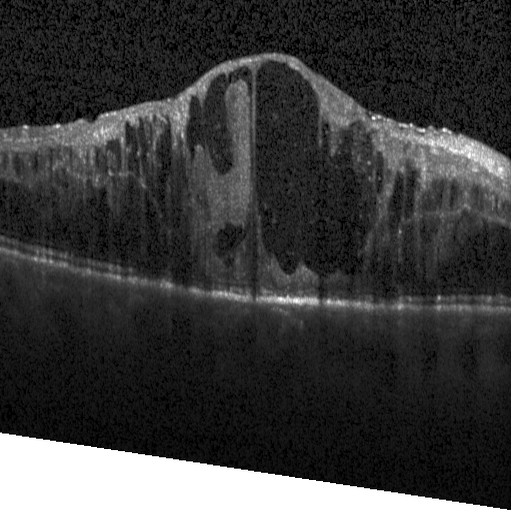

OCT finding: DME.